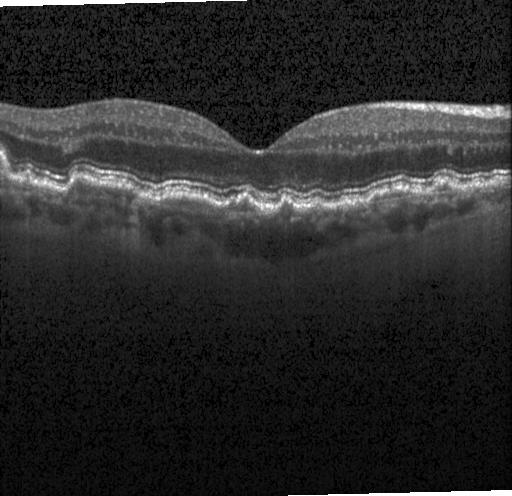
Assessment: multiple drusen.